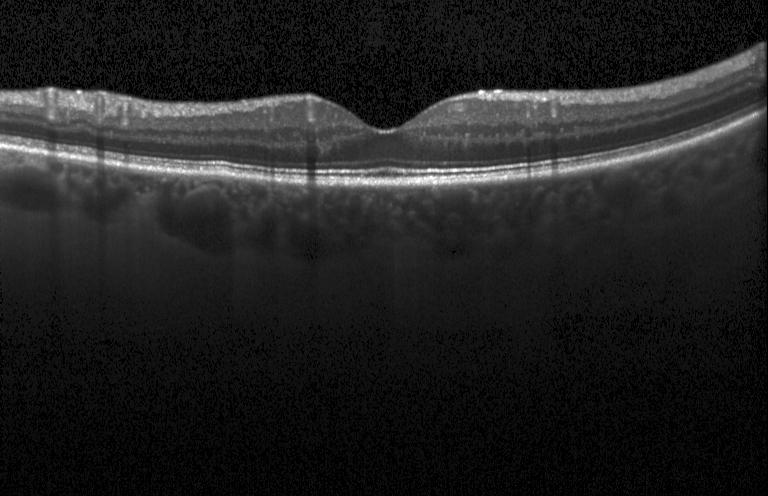

Finding: no evidence of CNV, DME, or drusen.